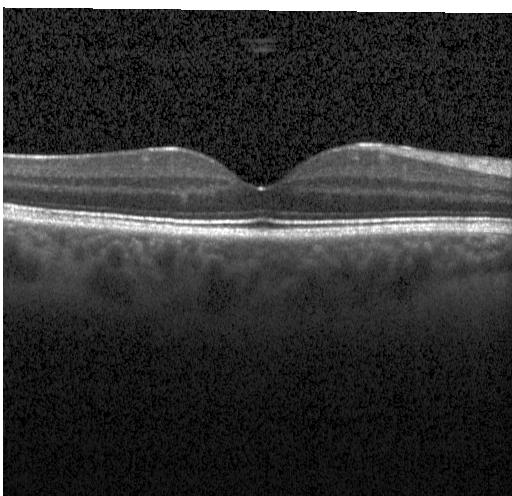 Retinal OCT cross-section, horizontal scan through the fovea
Diagnosis: no choroidal neovascularization, diabetic macular edema, or drusen.